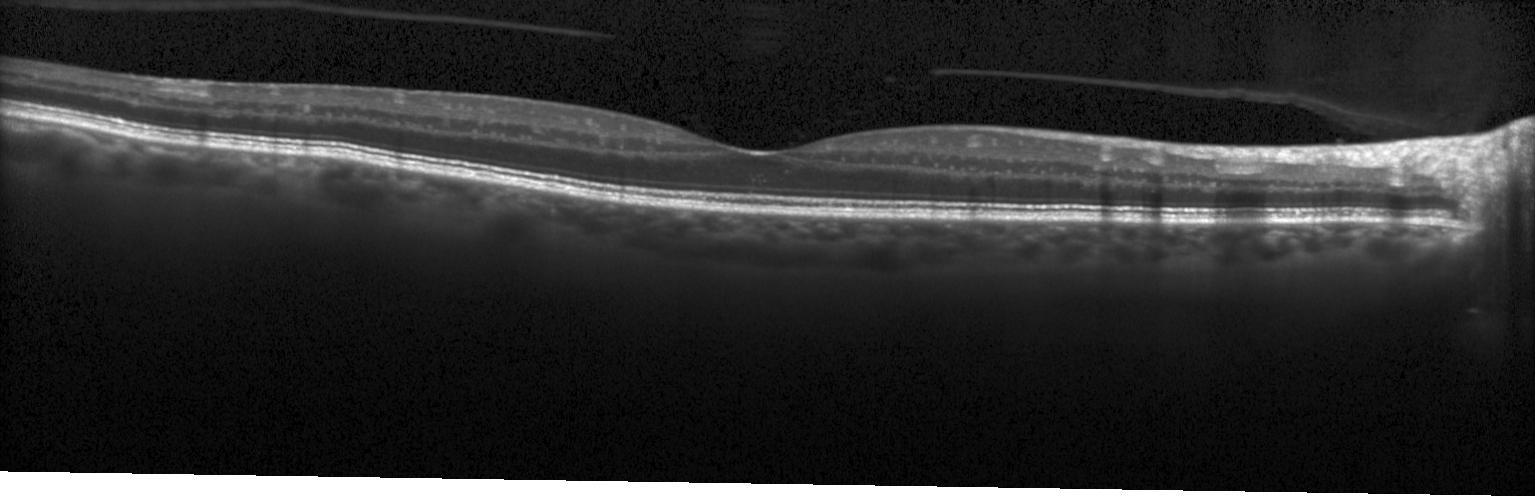 SD-OCT; acquired on a Heidelberg Spectralis; centered on the fovea; OCT line scan — Impression: neither choroidal neovascularization, diabetic macular edema, nor drusen.